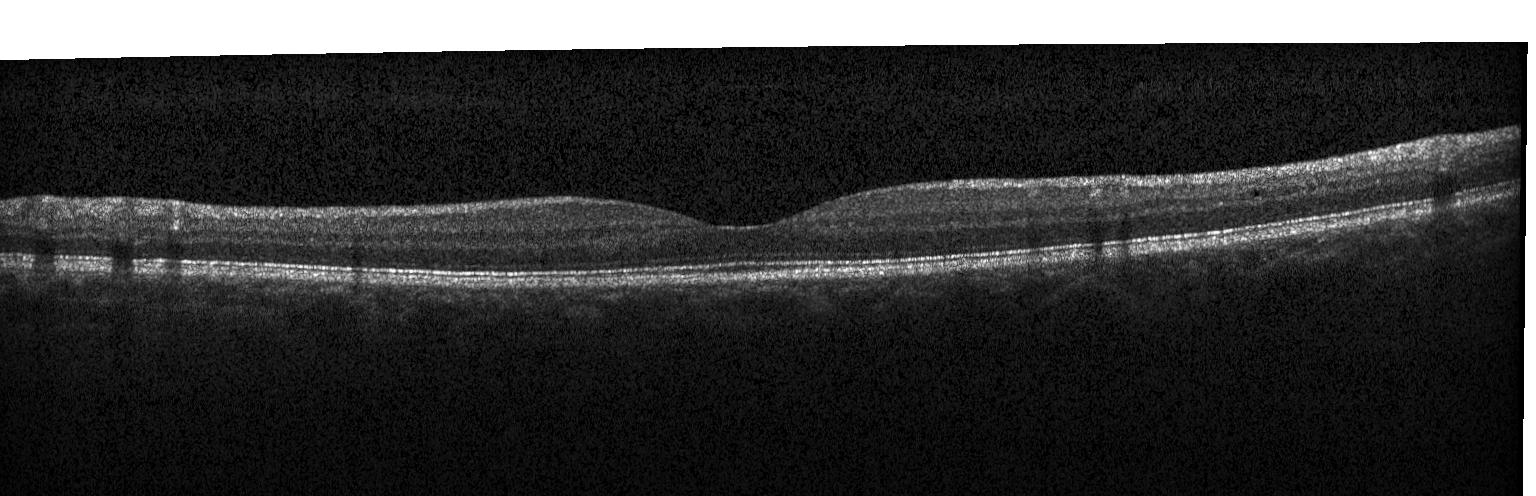

Diagnosis: no evidence of choroidal neovascularization, diabetic macular edema, or drusen.